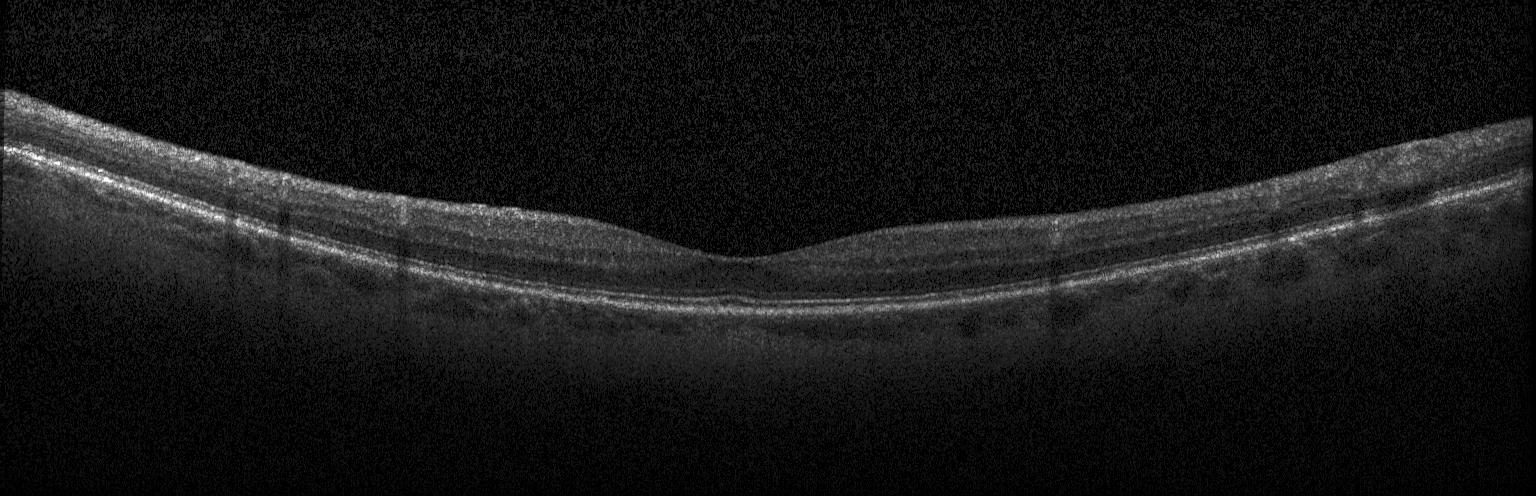
Heidelberg Spectralis · retinal OCT B-scan · fovea-centered
No evidence of choroidal neovascularization, diabetic macular edema, or drusen.